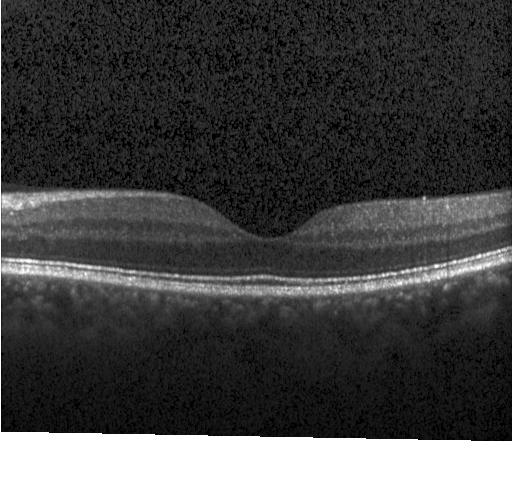
Optical coherence tomography scan; Heidelberg Spectralis OCT system.
Macular OCT: neither choroidal neovascularization, diabetic macular edema, nor drusen.